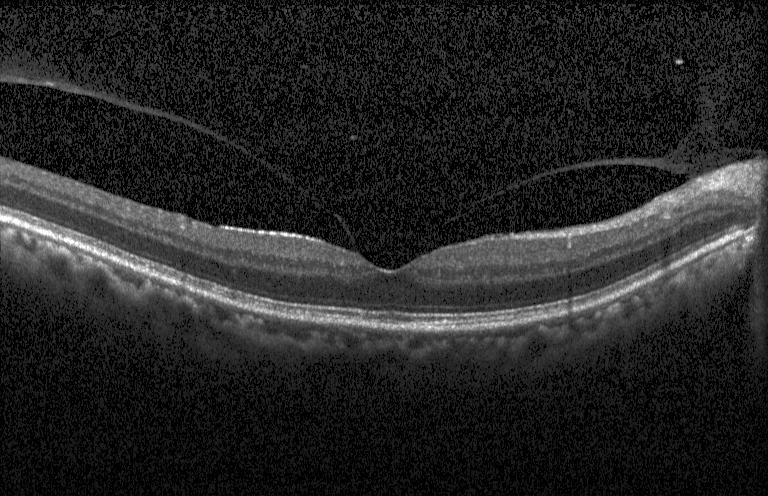
SD-OCT, Heidelberg Spectralis, OCT line scan — This B-scan demonstrates no evidence of choroidal neovascularization, diabetic macular edema, or drusen.